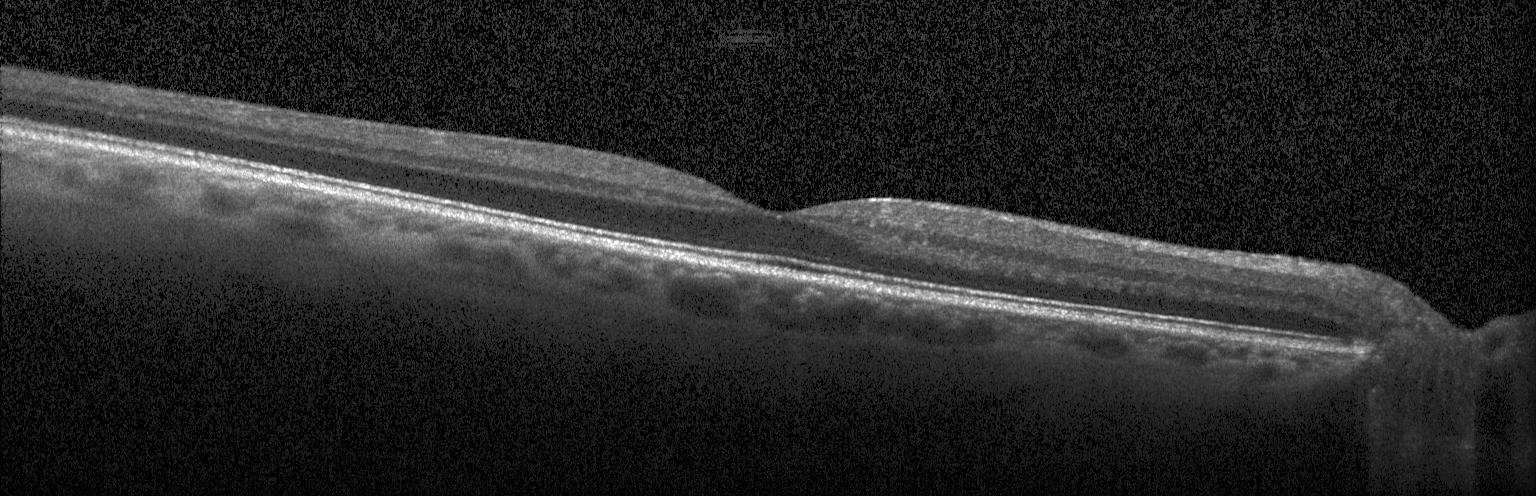
Optical coherence tomography B-scan; spectral-domain OCT; macular scan; Heidelberg Spectralis OCT system. The scan shows no choroidal neovascularization, no diabetic macular edema, and no drusen.